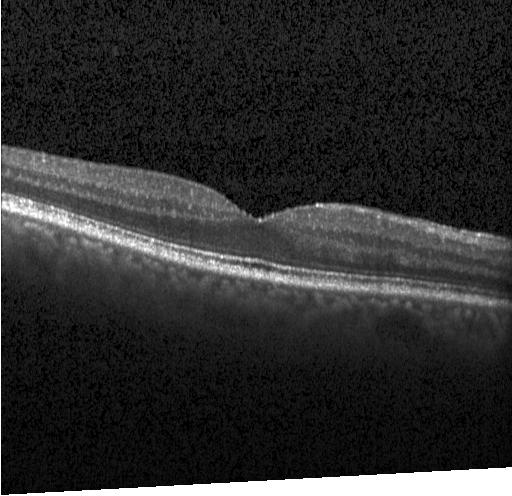

Fovea-centered; retinal OCT cross-section; Heidelberg Spectralis
The scan shows no evidence of choroidal neovascularization, diabetic macular edema, or drusen.